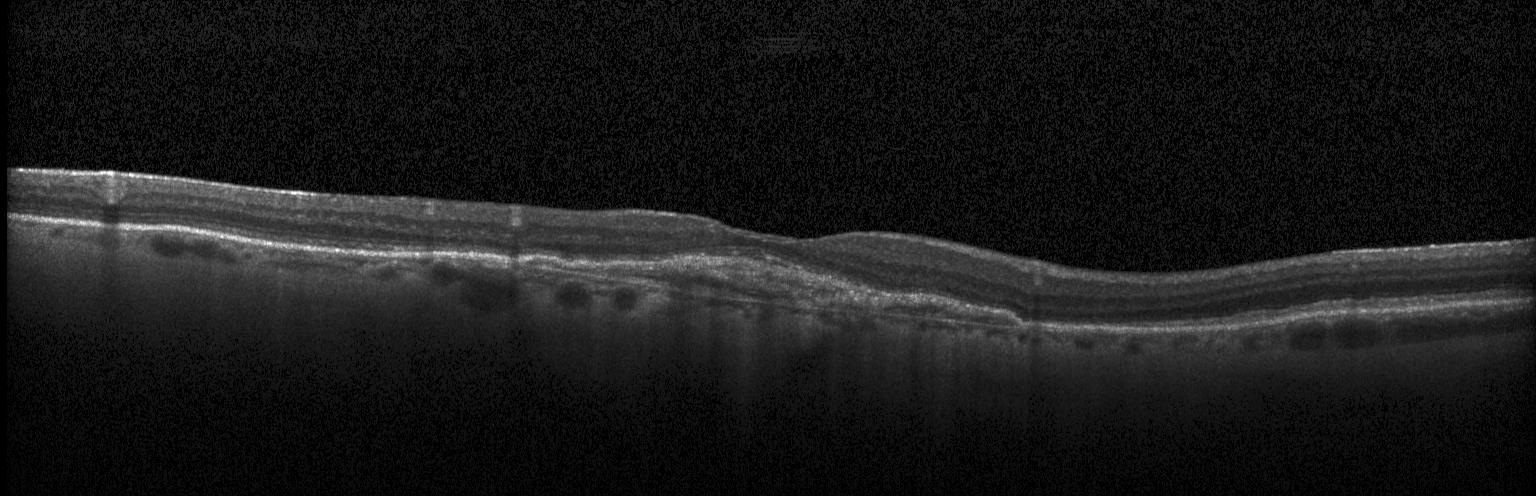

Diagnosis: a choroidal neovascular membrane.